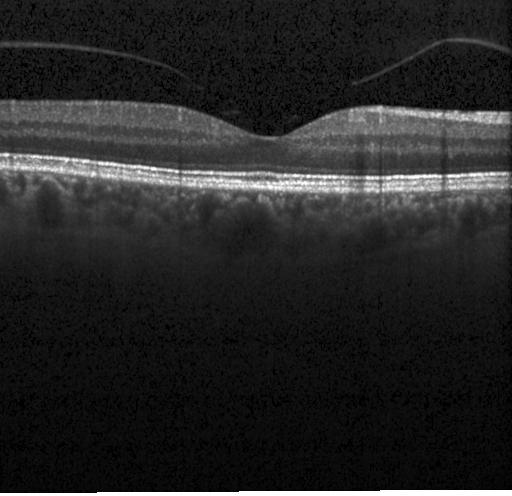
Finding: no CNV, DME, or drusen.